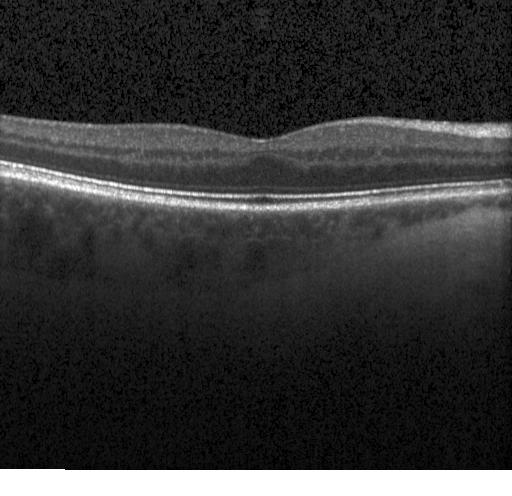 Optical coherence tomography scan — Impression: neither choroidal neovascularization, diabetic macular edema, nor drusen.